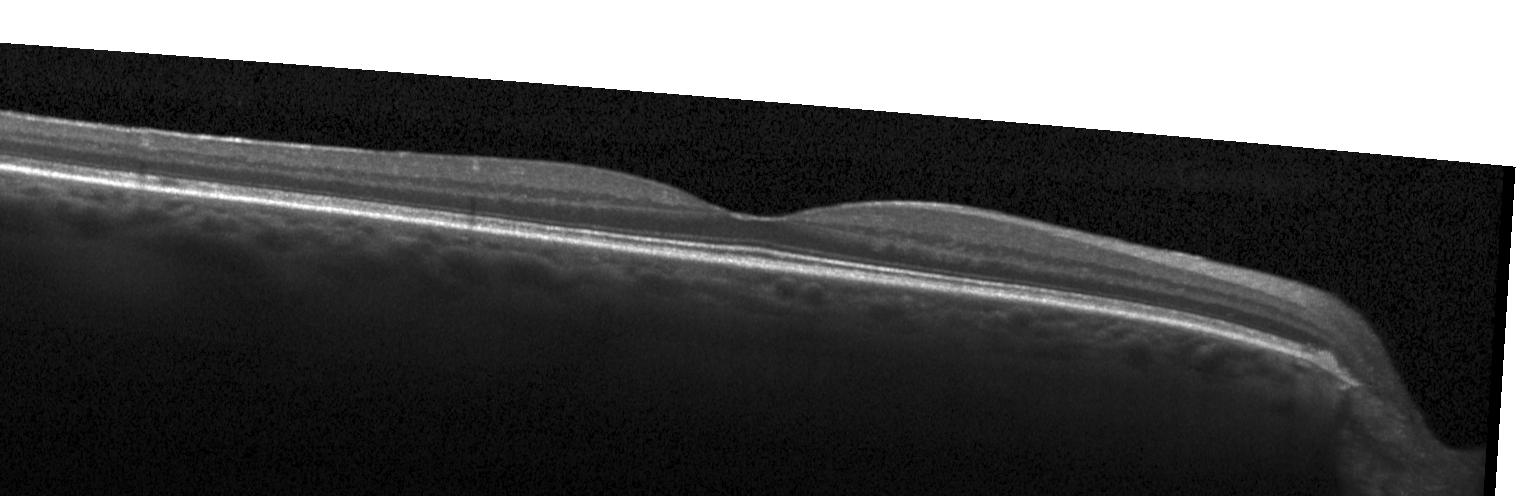
Acquired on a Heidelberg Spectralis · retinal OCT cross-section
No choroidal neovascularization, no diabetic macular edema, and no drusen.